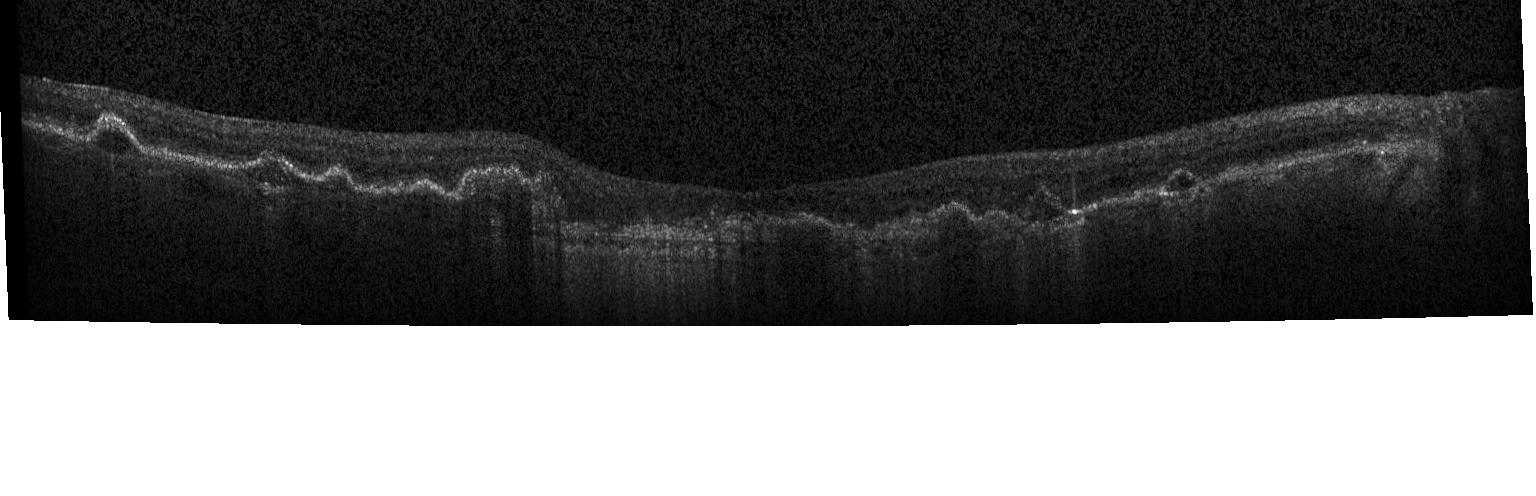
Spectral-domain OCT. OCT B-scan — This B-scan demonstrates a choroidal neovascular membrane.